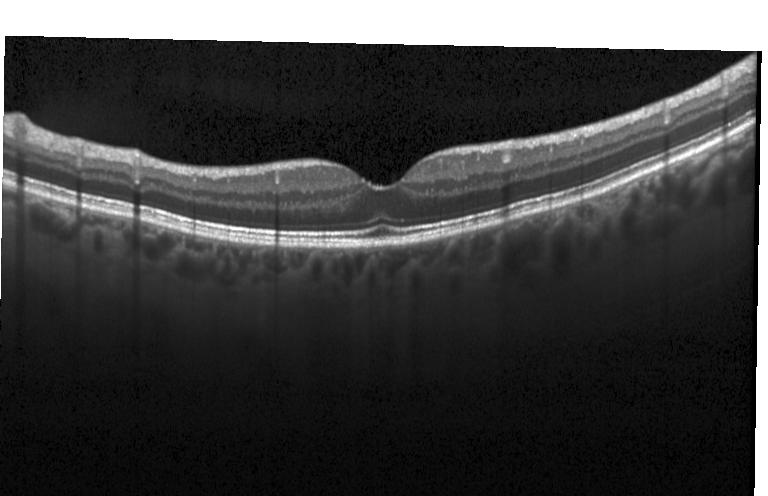
No evidence of CNV, DME, or drusen.